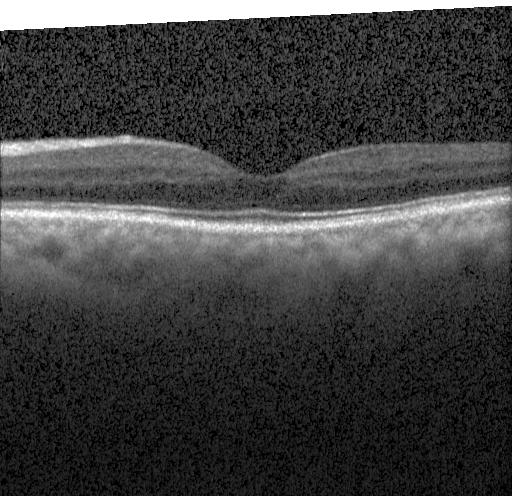
Optical coherence tomography scan.
The scan shows no choroidal neovascularization, no diabetic macular edema, and no drusen.